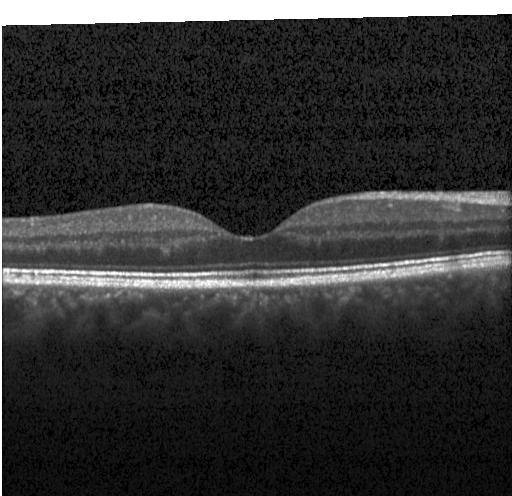 Impression: no choroidal neovascularization, no diabetic macular edema, and no drusen.